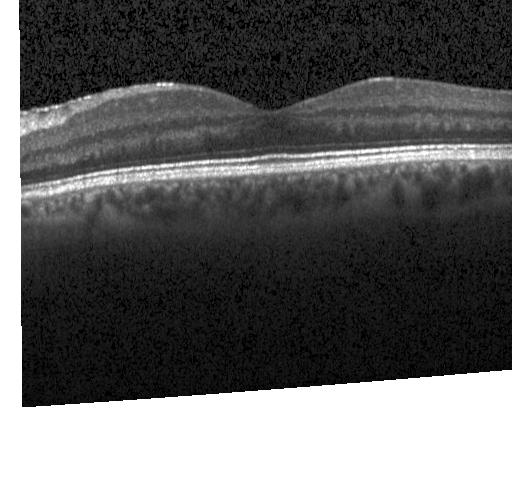
Finding: no CNV, DME, or drusen.